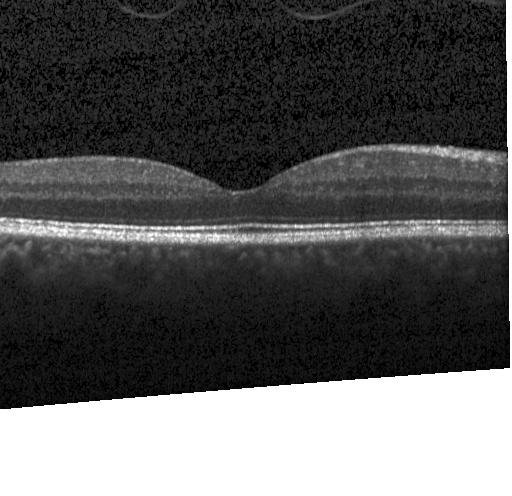

OCT B-scan. Heidelberg Spectralis. Spectral-domain optical coherence tomography
Finding: no CNV, no DME, and no drusen.